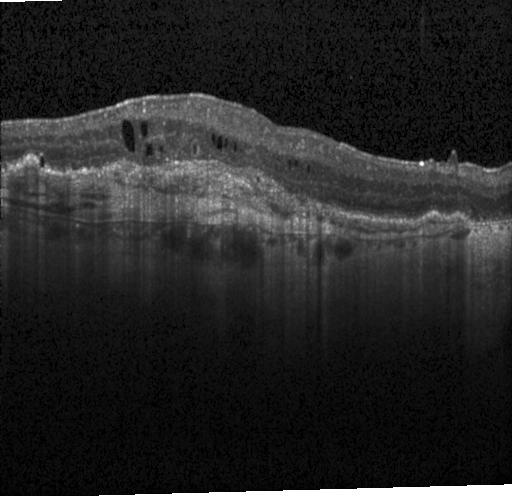

Optical coherence tomography scan. A choroidal neovascular membrane.